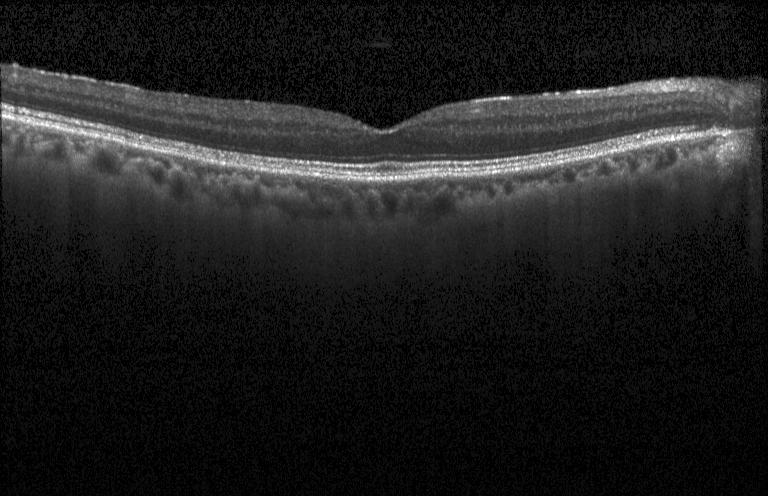 The scan shows no choroidal neovascularization, diabetic macular edema, or drusen.